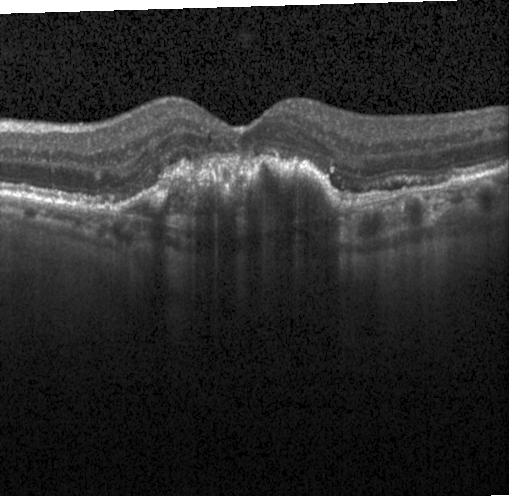

Macular OCT: choroidal neovascularization (CNV).